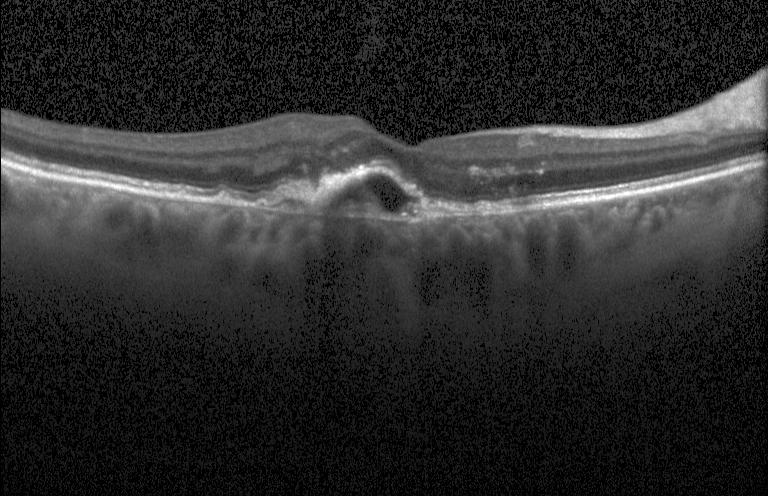
Spectral-domain OCT; OCT line scan; instrument: Heidelberg Spectralis; through the macula.
Diagnosis: choroidal neovascularization (CNV).